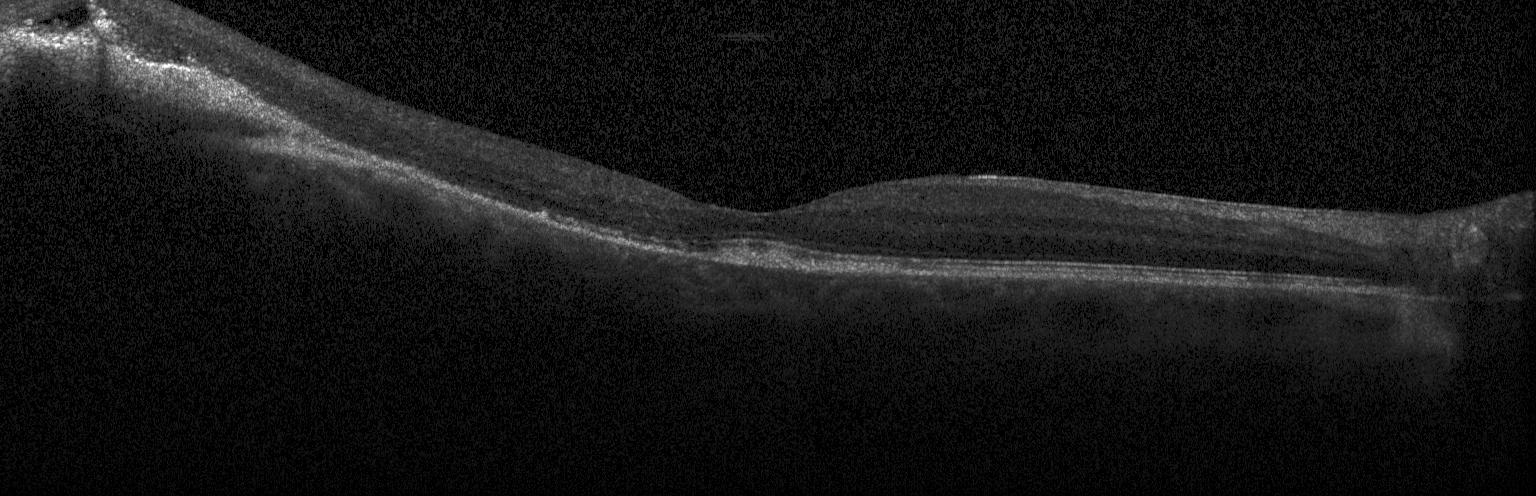 Heidelberg Spectralis. OCT line scan — Impression: choroidal neovascularization (CNV).